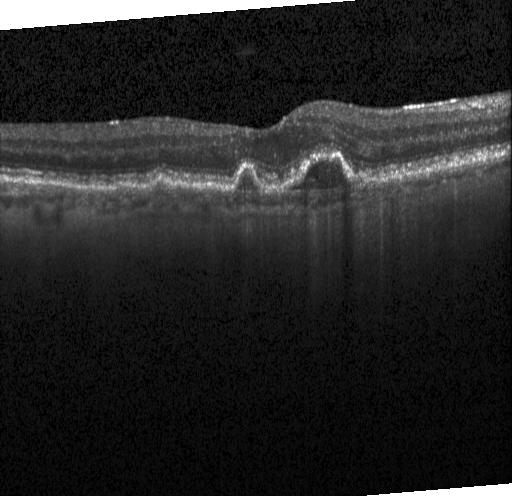 OCT finding: choroidal neovascularization (CNV).